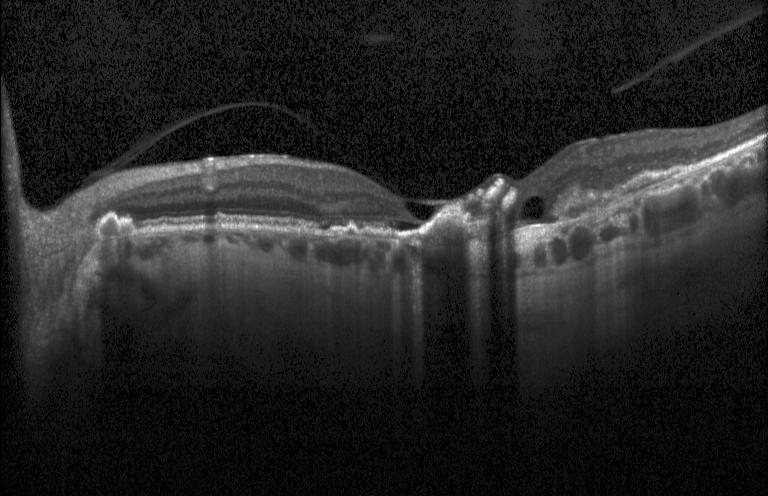

Optical coherence tomography scan, through the macula, SD-OCT, Heidelberg Spectralis. Finding: choroidal neovascularization.